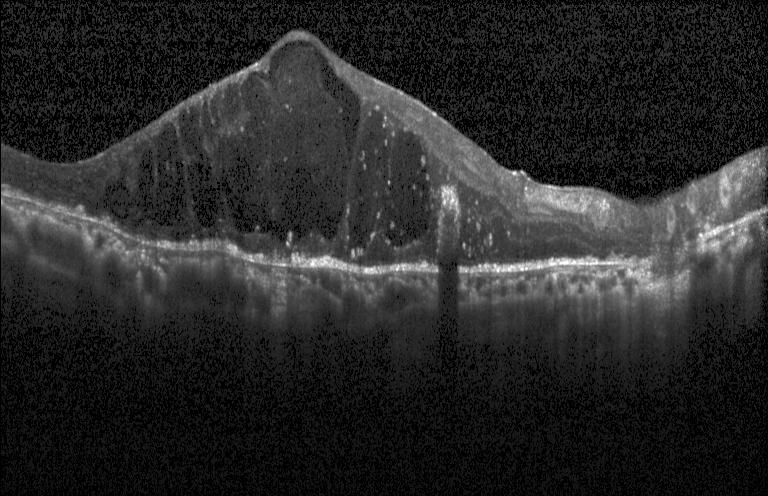 Optical coherence tomography B-scan.
Macular OCT: DME.